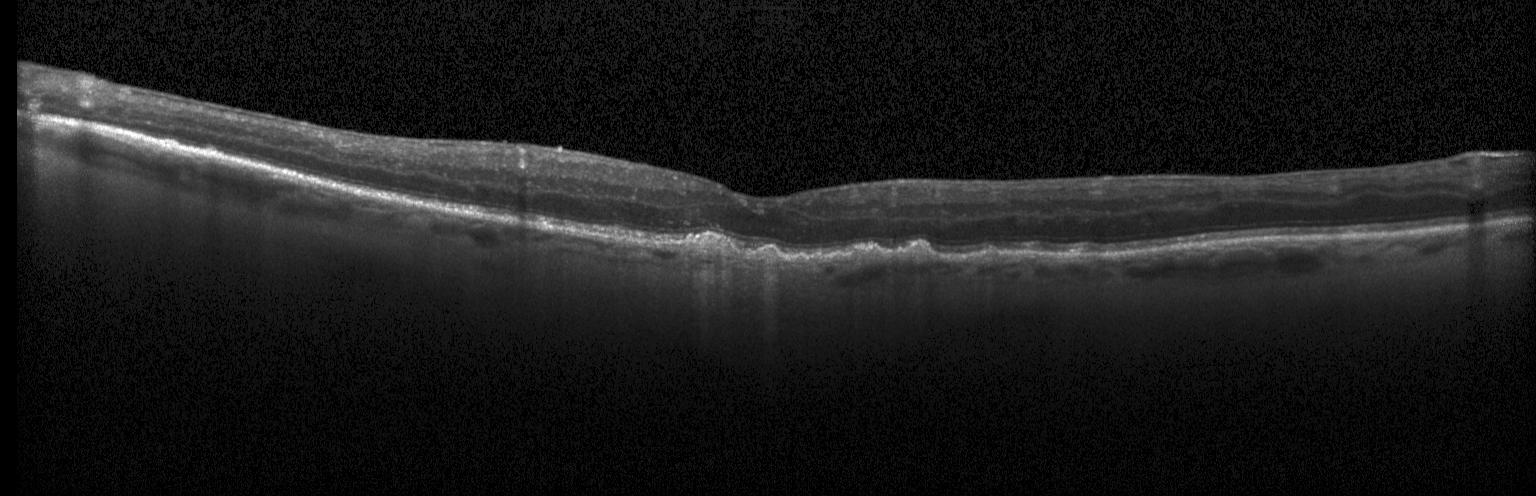 Centered on the fovea. Retinal OCT B-scan. Heidelberg Spectralis OCT system
The scan shows CNV.